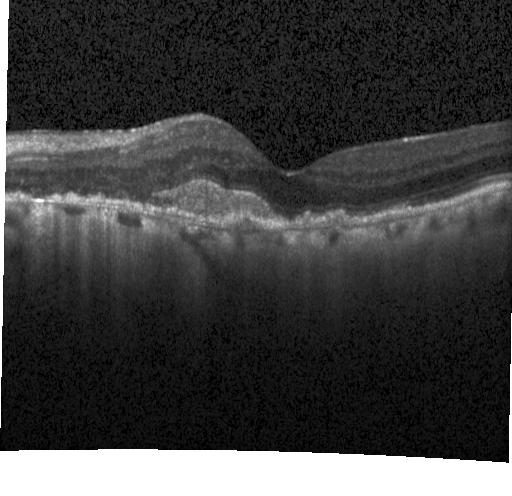

OCT B-scan. Finding: choroidal neovascularization.